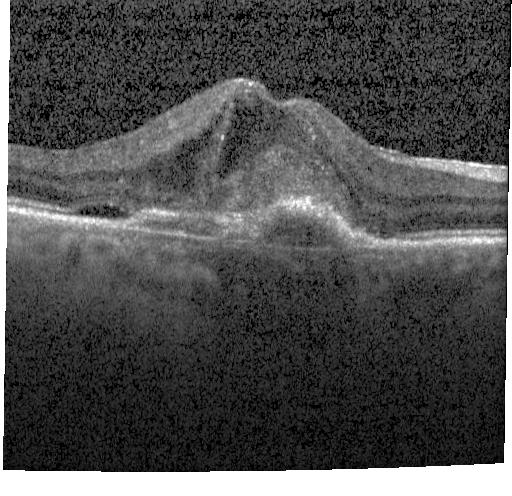 Heidelberg Spectralis; spectral-domain optical coherence tomography; optical coherence tomography B-scan
Diagnosis: a choroidal neovascular membrane.